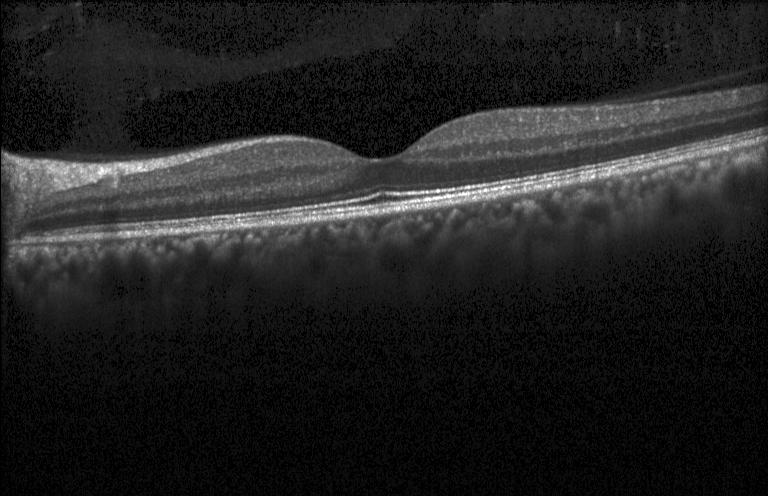 Retinal OCT cross-section; Heidelberg Spectralis.
Finding: no CNV, DME, or drusen.